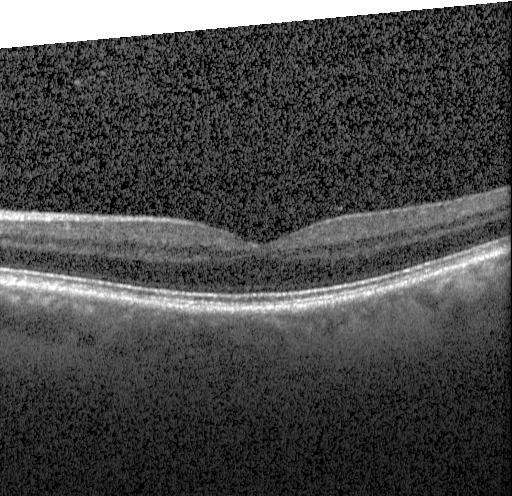
Retinal OCT B-scan
No choroidal neovascularization, diabetic macular edema, or drusen.